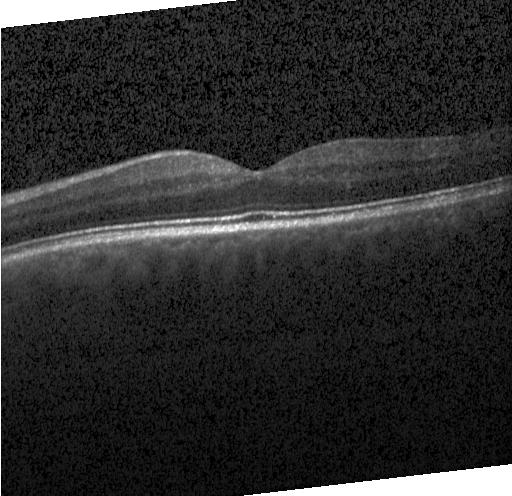 Spectral-domain OCT; Heidelberg Spectralis; optical coherence tomography scan; horizontal scan through the fovea
Impression: neither CNV, DME, nor drusen.